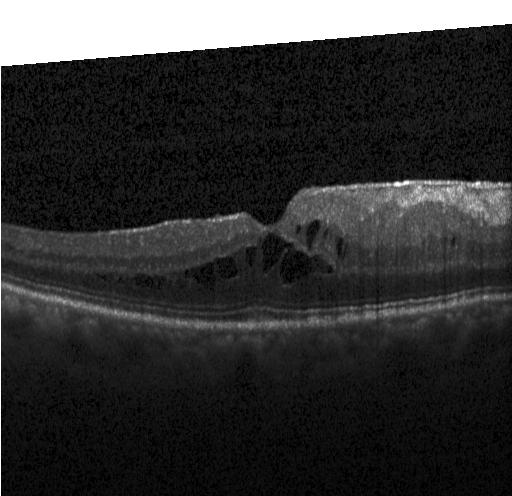 Instrument: Heidelberg Spectralis, OCT line scan, horizontal scan through the fovea.
This B-scan demonstrates DME.